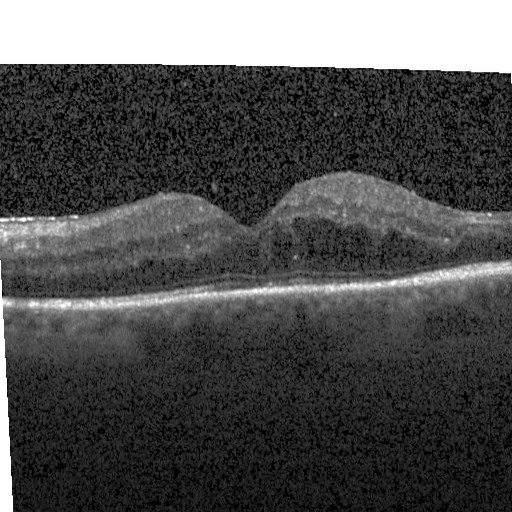

Retinal OCT B-scan.
Dx: diabetic macular edema.